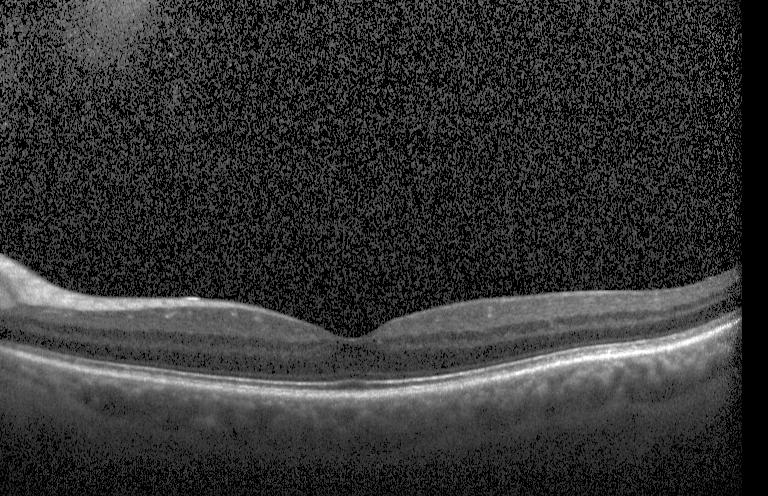 Retinal OCT cross-section showing neither choroidal neovascularization, diabetic macular edema, nor drusen.